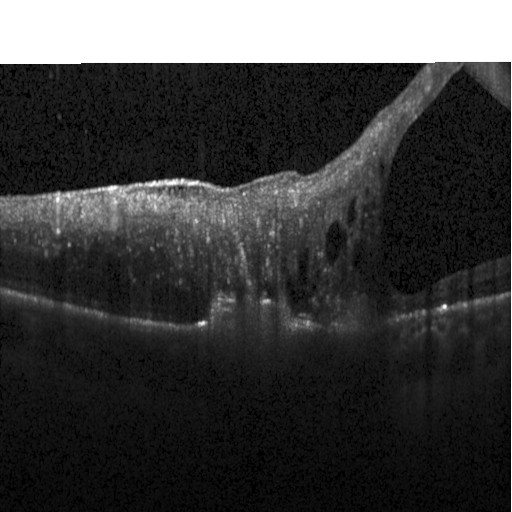
Diagnosis: diabetic macular edema.